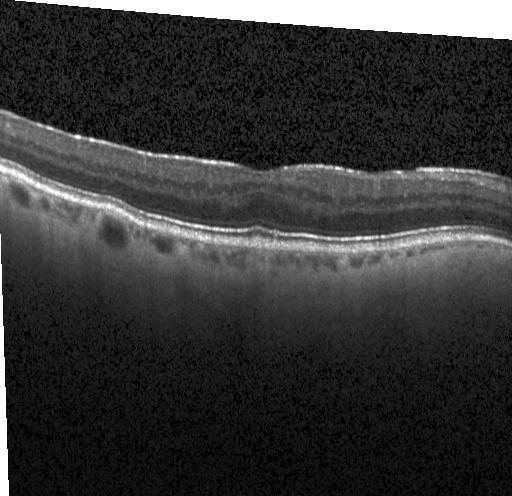
Retinal OCT cross-section. Spectral-domain optical coherence tomography — Macular OCT: sub-RPE drusenoid deposits.